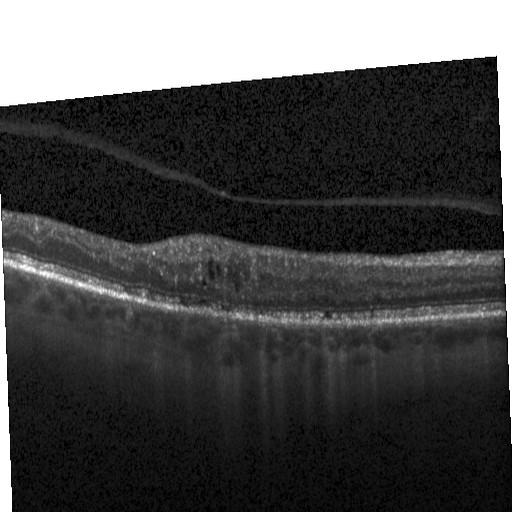

Retinal OCT cross-section showing diabetic macular edema.